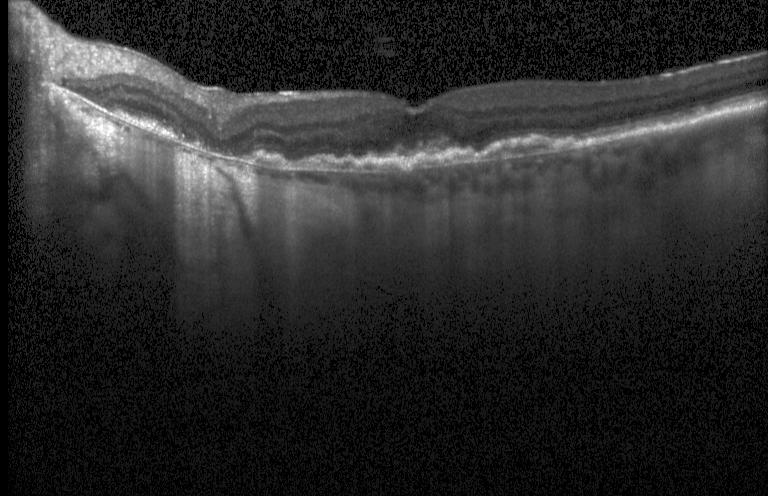
OCT B-scan
A choroidal neovascular membrane.